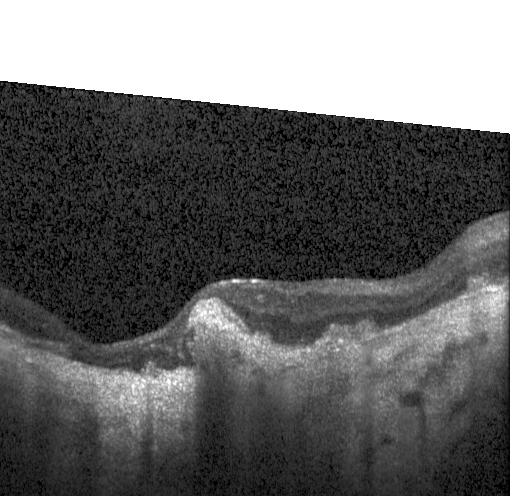

Diagnosis: a choroidal neovascular membrane.